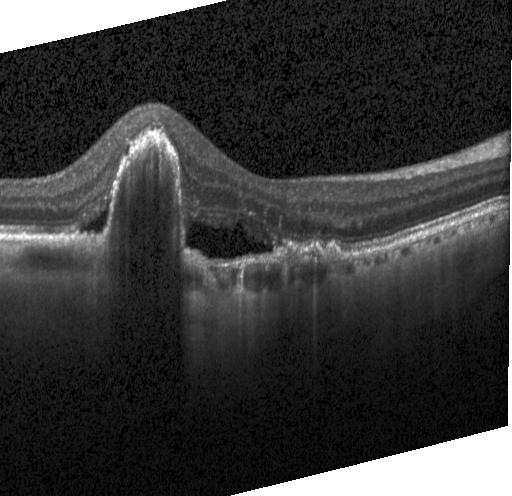

Finding: choroidal neovascularization (CNV).